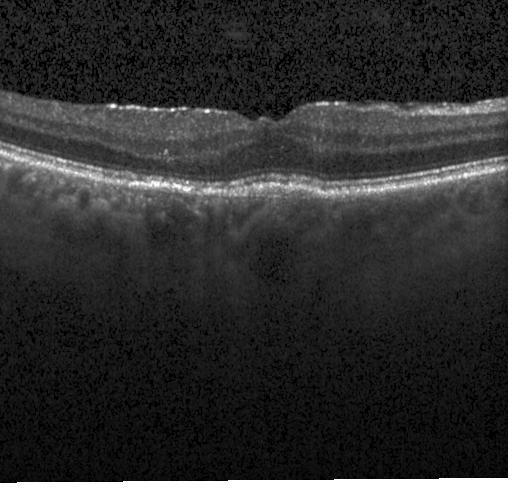 Acquired on a Heidelberg Spectralis. Fovea-centered. Retinal OCT cross-section
Finding: CNV.